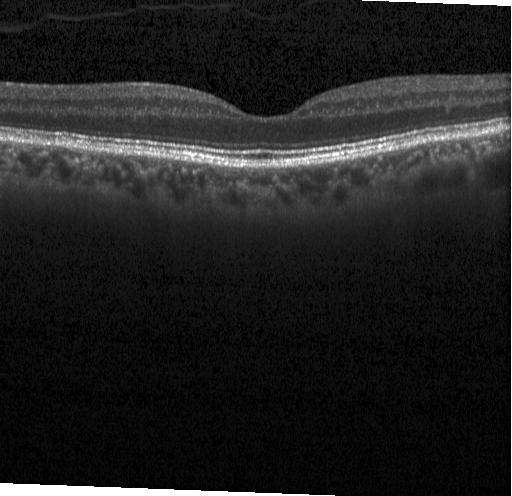

Optical coherence tomography scan · horizontal scan through the fovea · acquired on a Heidelberg Spectralis · spectral-domain optical coherence tomography. Finding: no CNV, no DME, and no drusen.